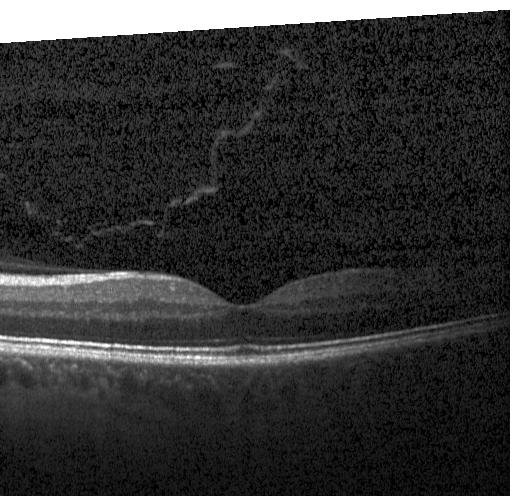
Horizontal scan through the fovea; retinal OCT B-scan; acquired on a Heidelberg Spectralis.
Impression: no evidence of choroidal neovascularization, diabetic macular edema, or drusen.